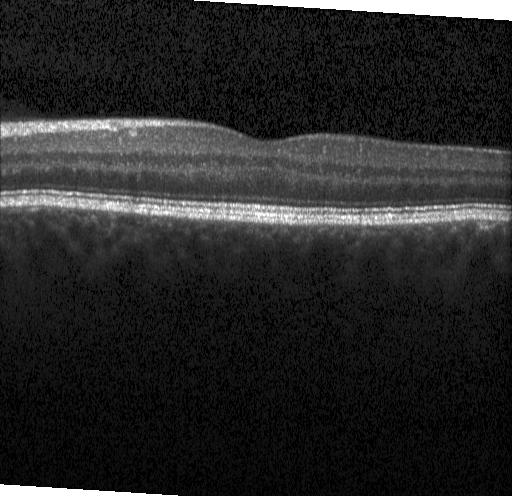
Spectral-domain OCT · OCT line scan
Macular OCT: no choroidal neovascularization, no diabetic macular edema, and no drusen.